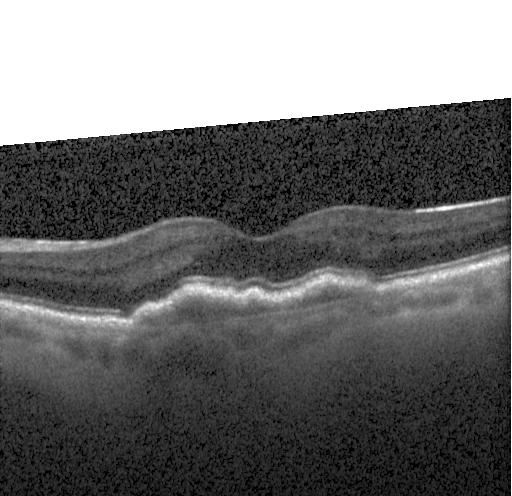

Dx: a choroidal neovascular membrane.